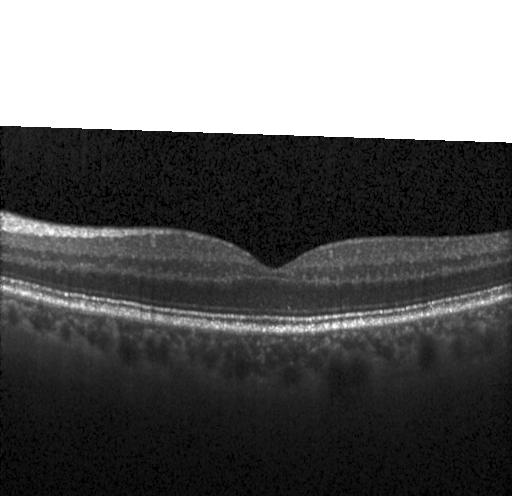
SD-OCT. Centered on the fovea. Heidelberg Spectralis. OCT B-scan — Impression: no choroidal neovascularization, diabetic macular edema, or drusen.